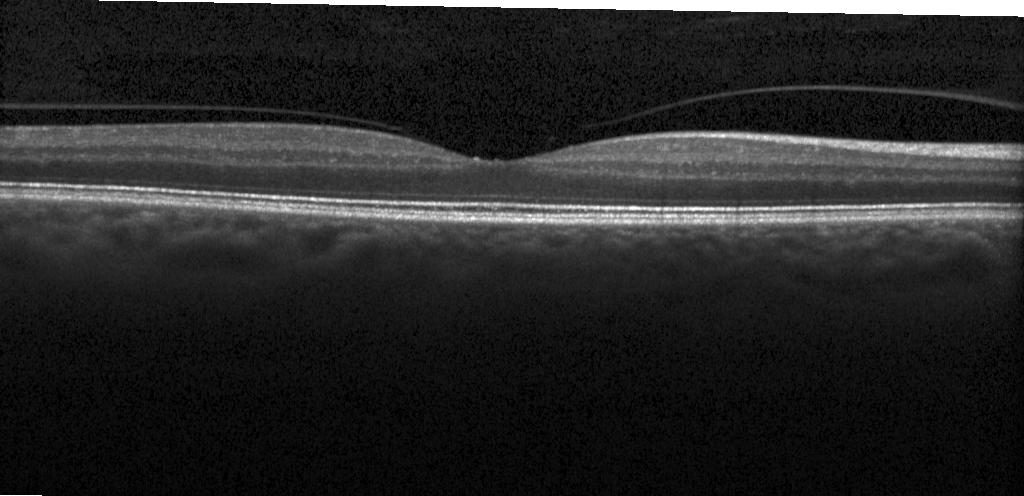
Dx: no choroidal neovascularization, no diabetic macular edema, and no drusen.